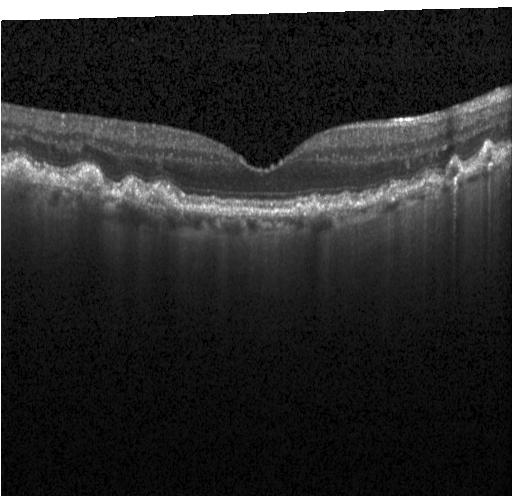 Fovea-centered. Optical coherence tomography B-scan. Spectral-domain optical coherence tomography. Acquired on a Heidelberg Spectralis. Impression: drusen.